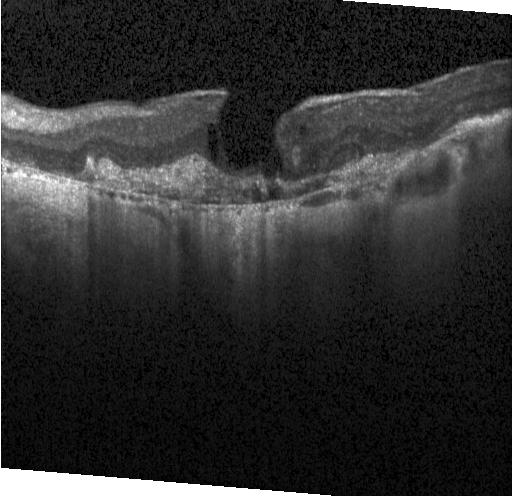 Assessment: a choroidal neovascular membrane.